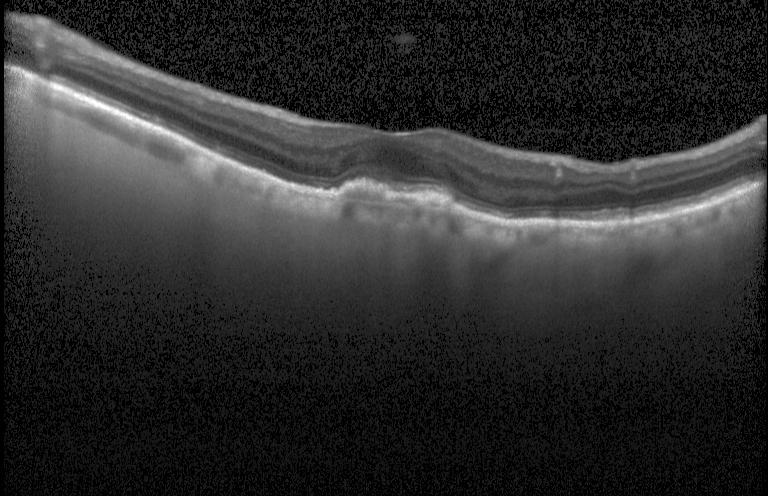 Diagnosis: a choroidal neovascular membrane.